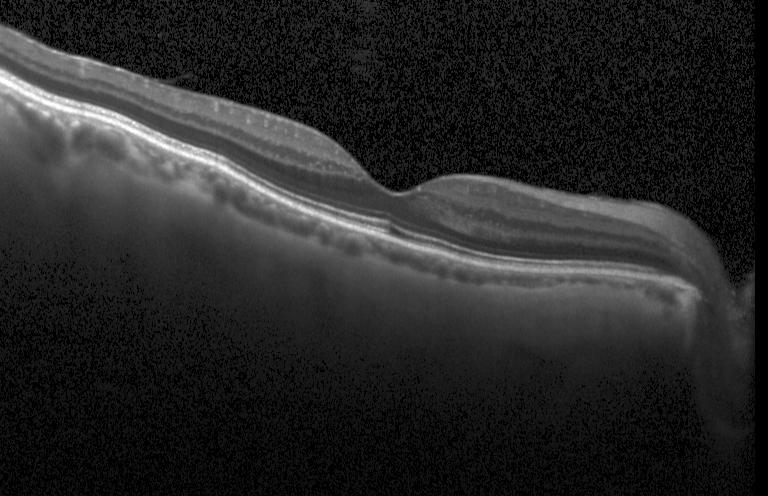
Retinal OCT B-scan · Heidelberg Spectralis
The scan shows no CNV, no DME, and no drusen.